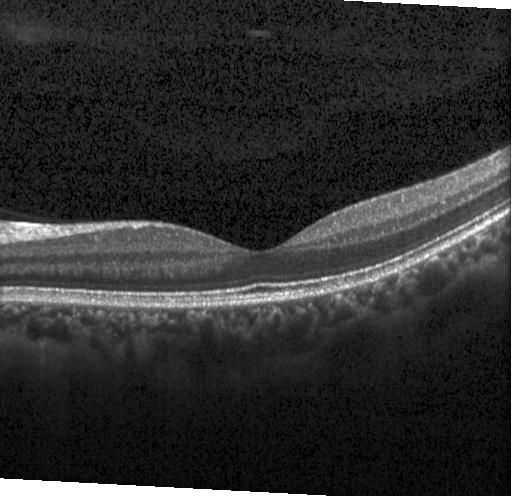
Acquired on a Heidelberg Spectralis, retinal OCT B-scan. Finding: neither choroidal neovascularization, diabetic macular edema, nor drusen.